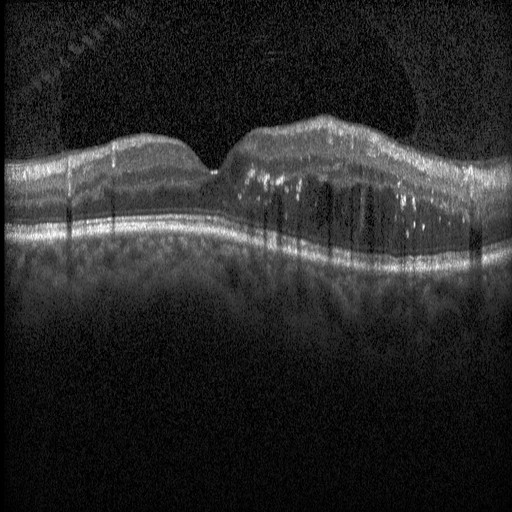
Instrument: Heidelberg Spectralis. Spectral-domain optical coherence tomography. Optical coherence tomography B-scan. Through the macula.
Finding: diabetic macular edema (DME).